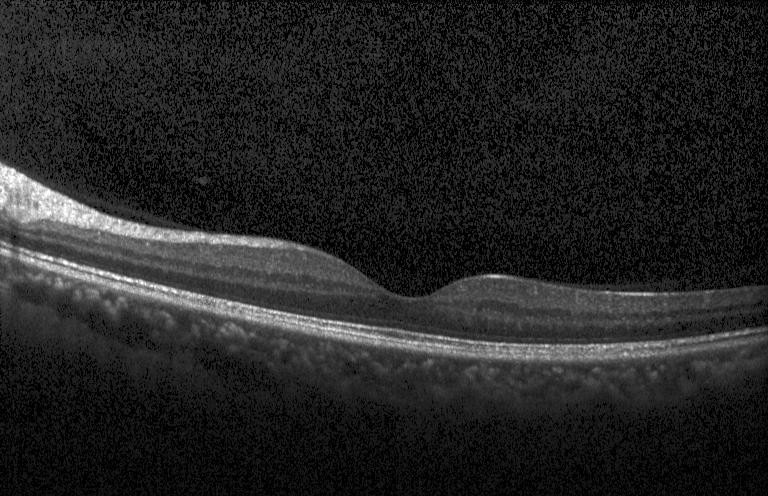 Spectral-domain optical coherence tomography · optical coherence tomography scan · instrument: Heidelberg Spectralis · horizontal scan through the fovea. Impression: neither CNV, DME, nor drusen.